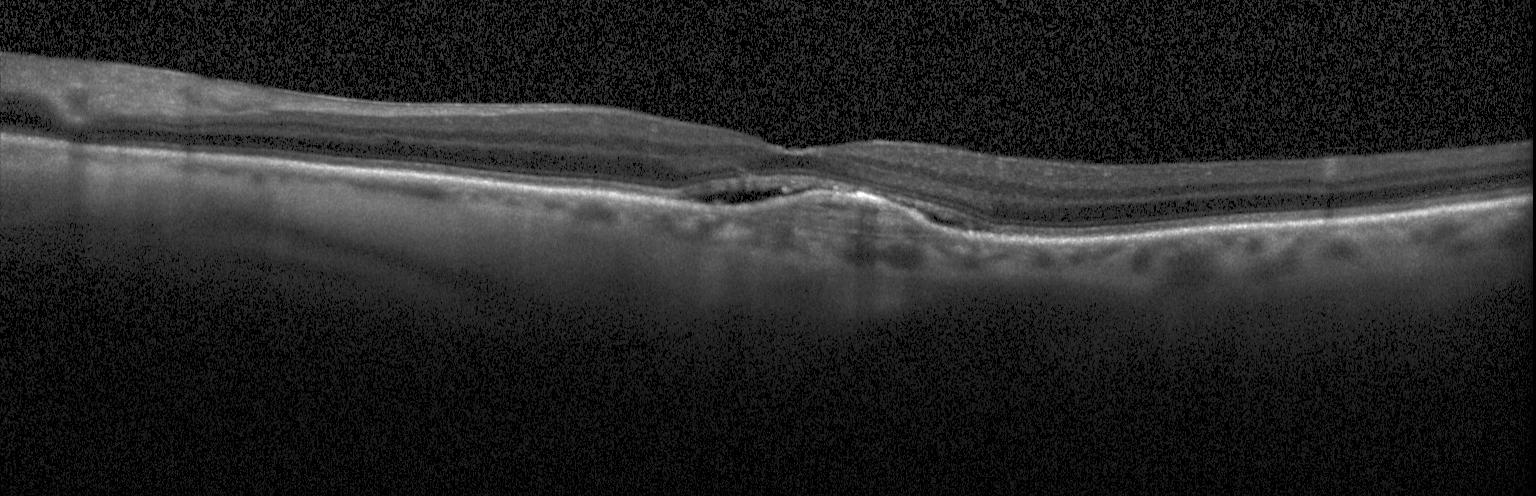 Retinal OCT B-scan; spectral-domain optical coherence tomography — A choroidal neovascular membrane.